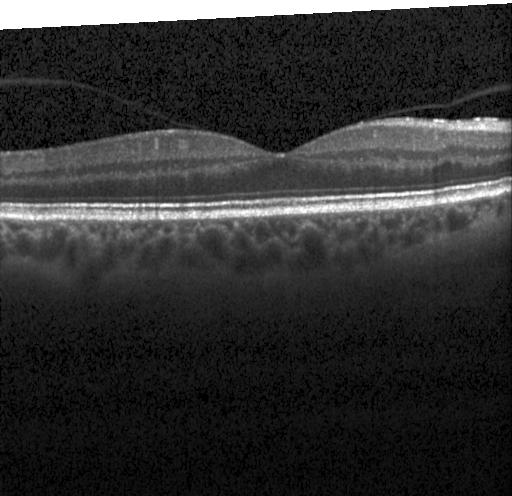

Optical coherence tomography B-scan, spectral-domain optical coherence tomography, Heidelberg Spectralis. No evidence of choroidal neovascularization, diabetic macular edema, or drusen.